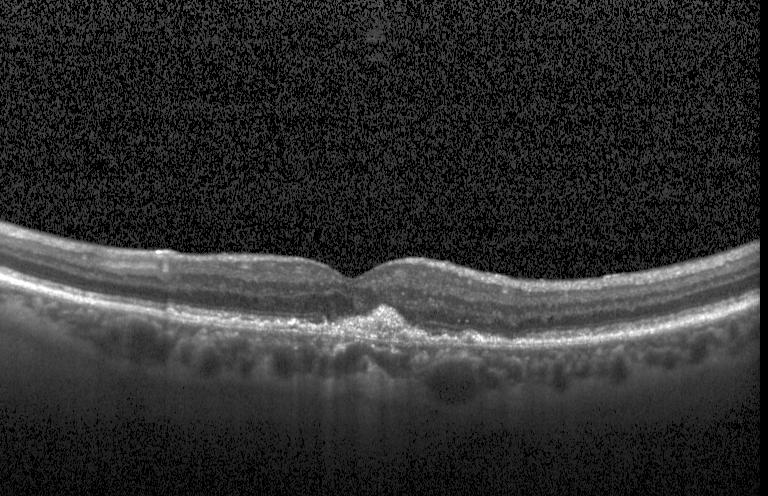
Finding: CNV.